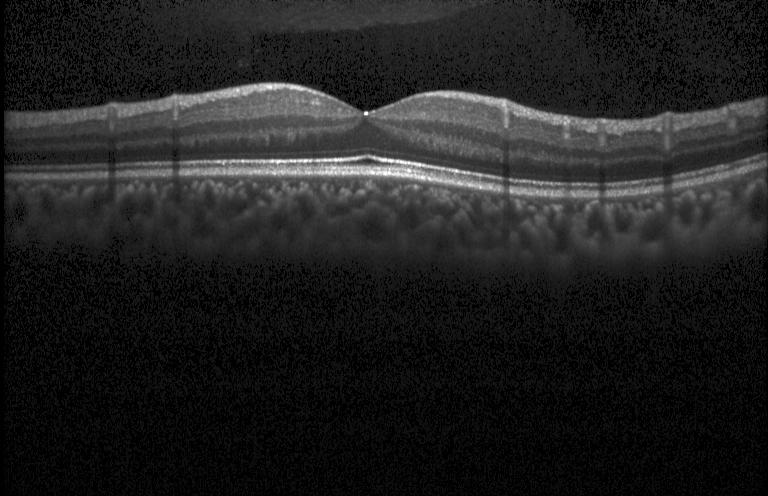

This B-scan demonstrates no evidence of choroidal neovascularization, diabetic macular edema, or drusen.